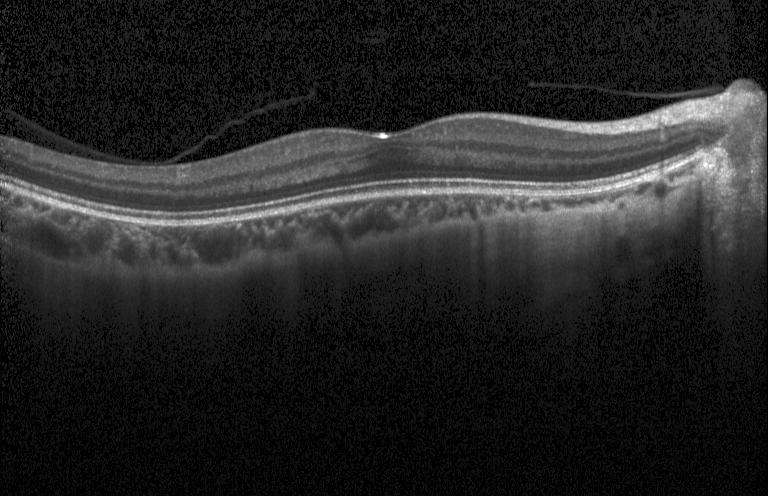

OCT B-scan. Spectral-domain optical coherence tomography.
Finding: neither choroidal neovascularization, diabetic macular edema, nor drusen.